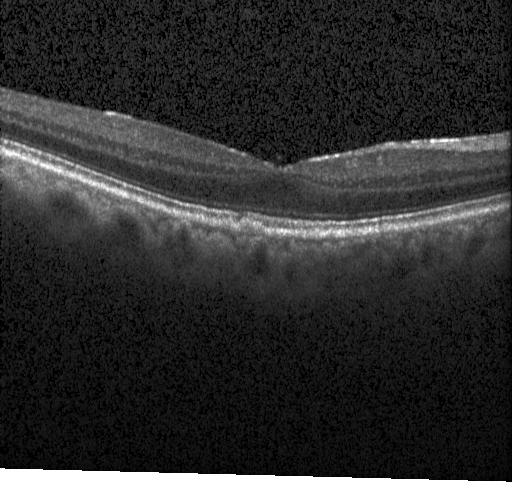 Heidelberg Spectralis. Fovea-centered. Retinal OCT cross-section. Spectral-domain optical coherence tomography — Impression: drusen.